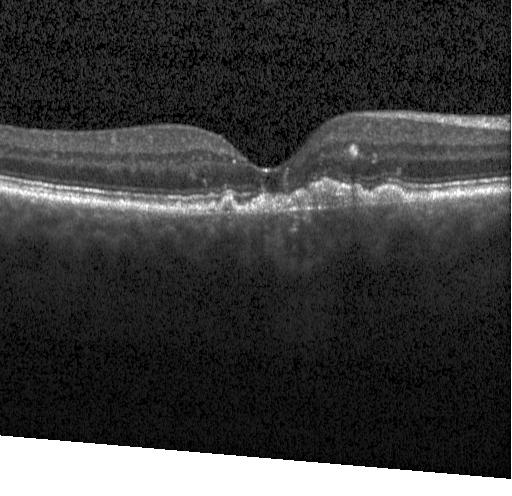 OCT line scan · through the macula · Heidelberg Spectralis. Diagnosis: a choroidal neovascular membrane.